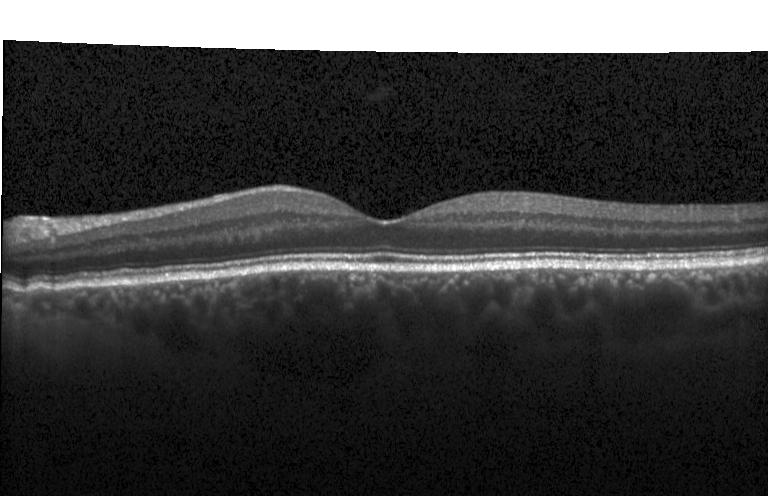
Optical coherence tomography B-scan. This B-scan demonstrates no choroidal neovascularization, no diabetic macular edema, and no drusen.